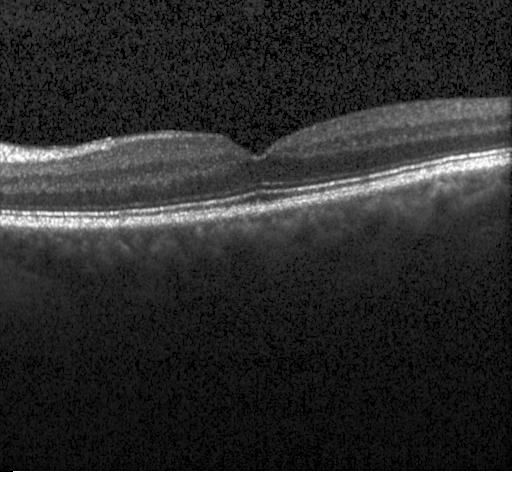

Macular OCT: no CNV, DME, or drusen.